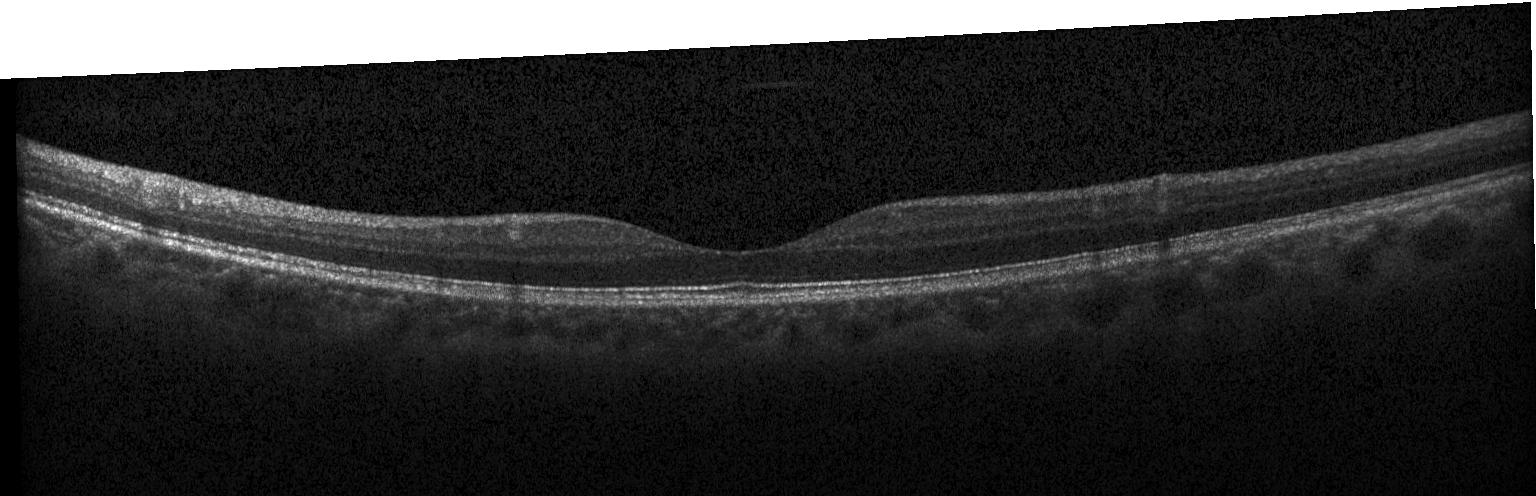 Spectral-domain OCT B-scan: no choroidal neovascularization, diabetic macular edema, or drusen.